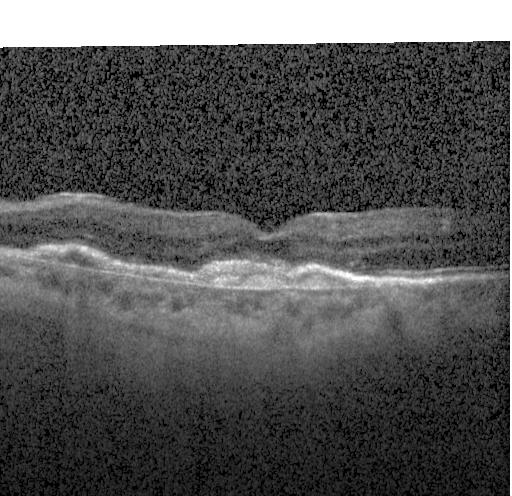

Instrument: Heidelberg Spectralis · OCT line scan.
OCT finding: a choroidal neovascular membrane.